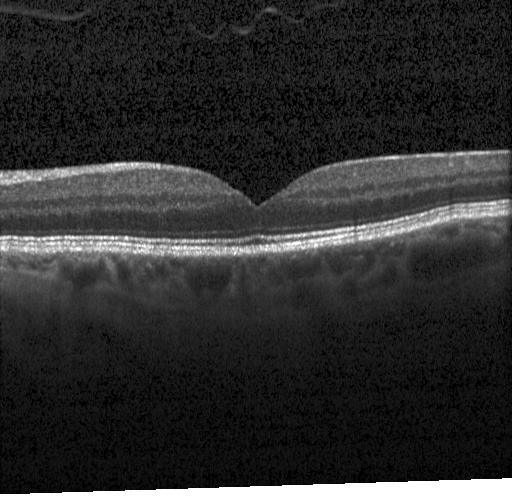
Optical coherence tomography scan — The scan shows neither choroidal neovascularization, diabetic macular edema, nor drusen.